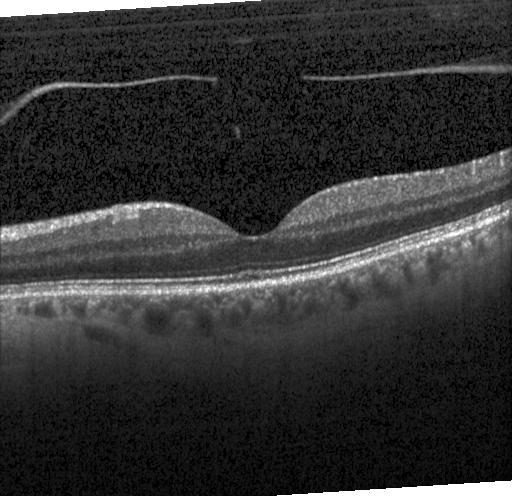 OCT scan showing no evidence of choroidal neovascularization, diabetic macular edema, or drusen.